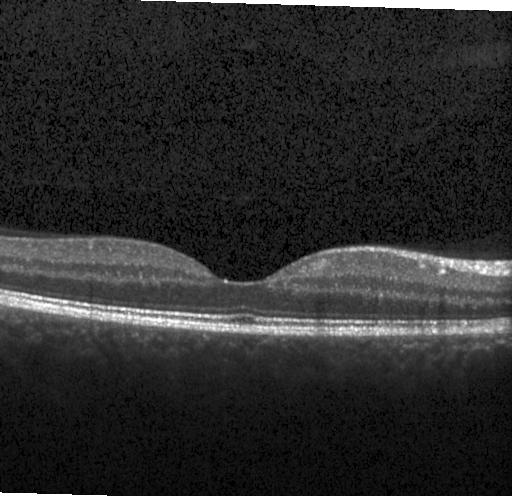

Optical coherence tomography scan, spectral-domain optical coherence tomography
The scan shows no CNV, DME, or drusen.